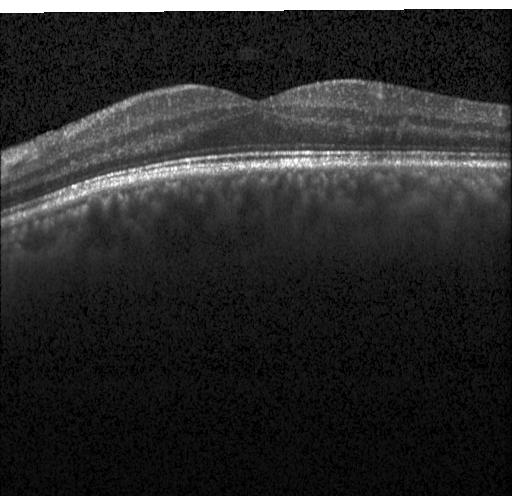

OCT B-scan showing no evidence of CNV, DME, or drusen.